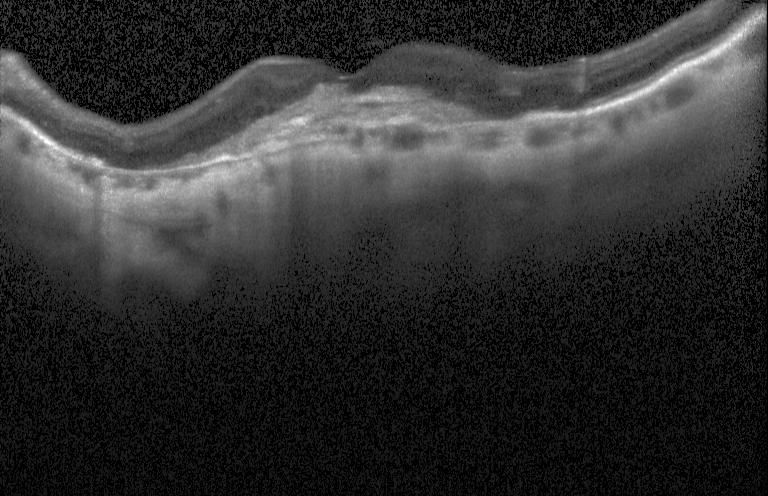

CNV.